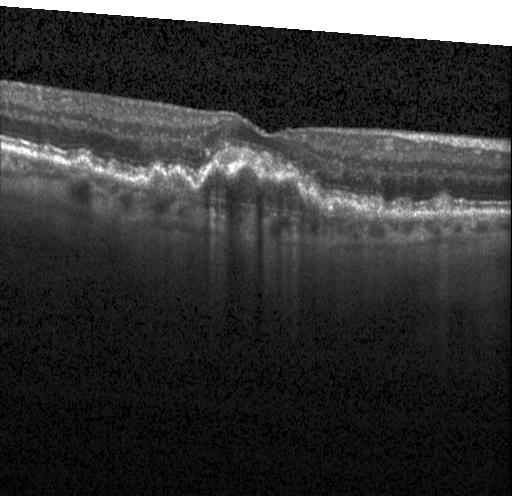

Macular OCT: choroidal neovascularization.